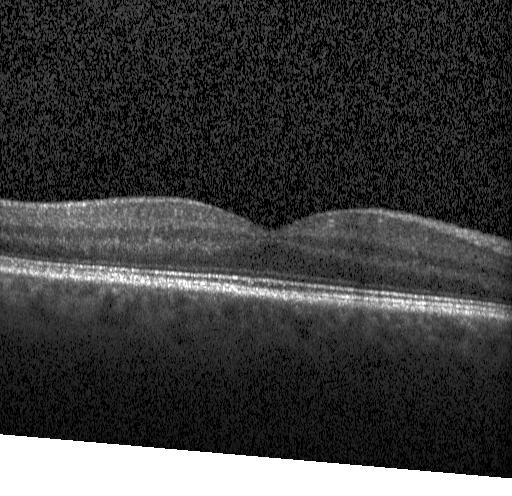

Retinal OCT cross-section showing no CNV, DME, or drusen.